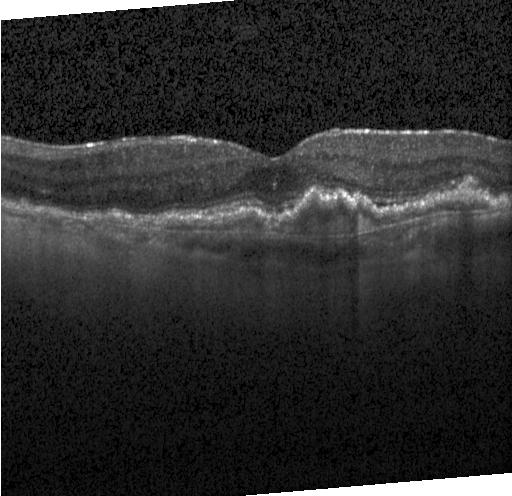

OCT B-scan showing CNV.